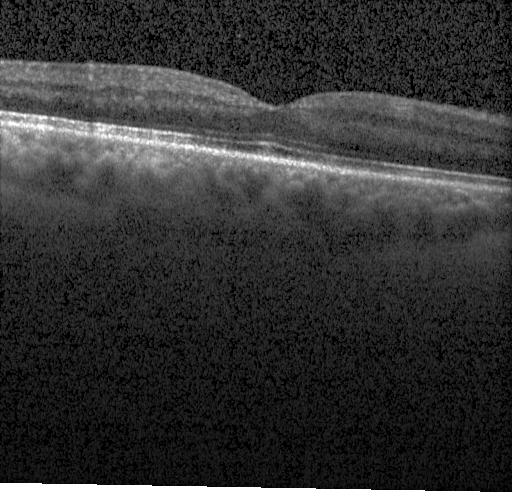

Retinal OCT B-scan — Impression: no choroidal neovascularization, no diabetic macular edema, and no drusen.